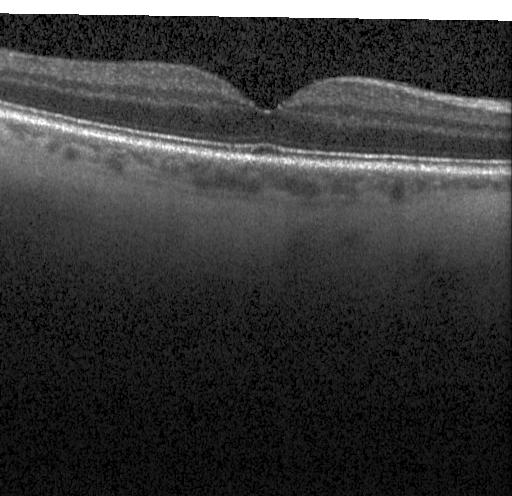 Neither choroidal neovascularization, diabetic macular edema, nor drusen.